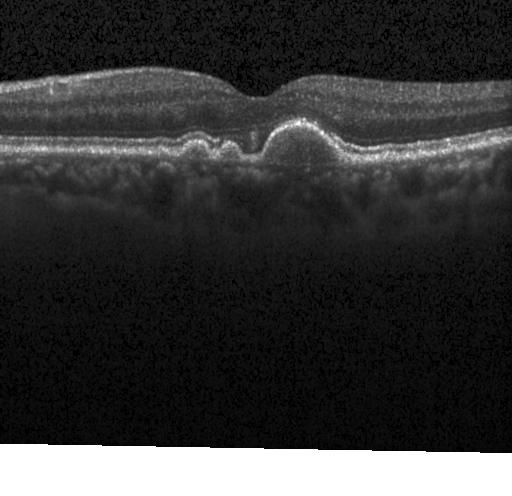 Macular OCT: sub-RPE drusenoid deposits.